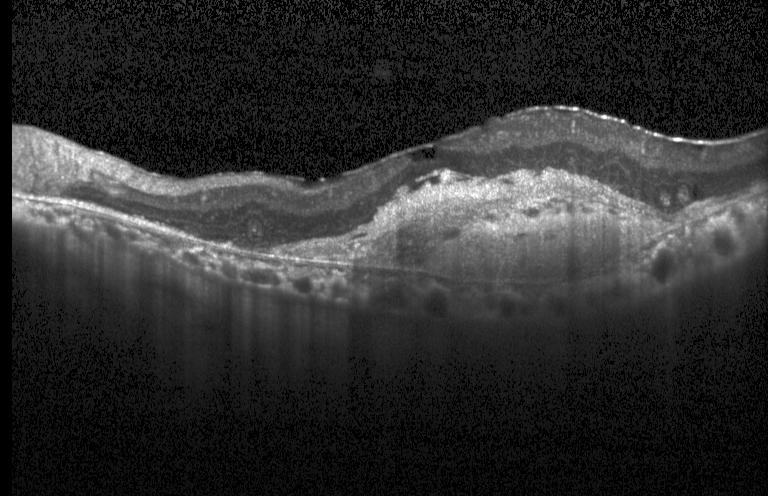

Heidelberg Spectralis; retinal OCT cross-section; macular scan — This B-scan demonstrates choroidal neovascularization.